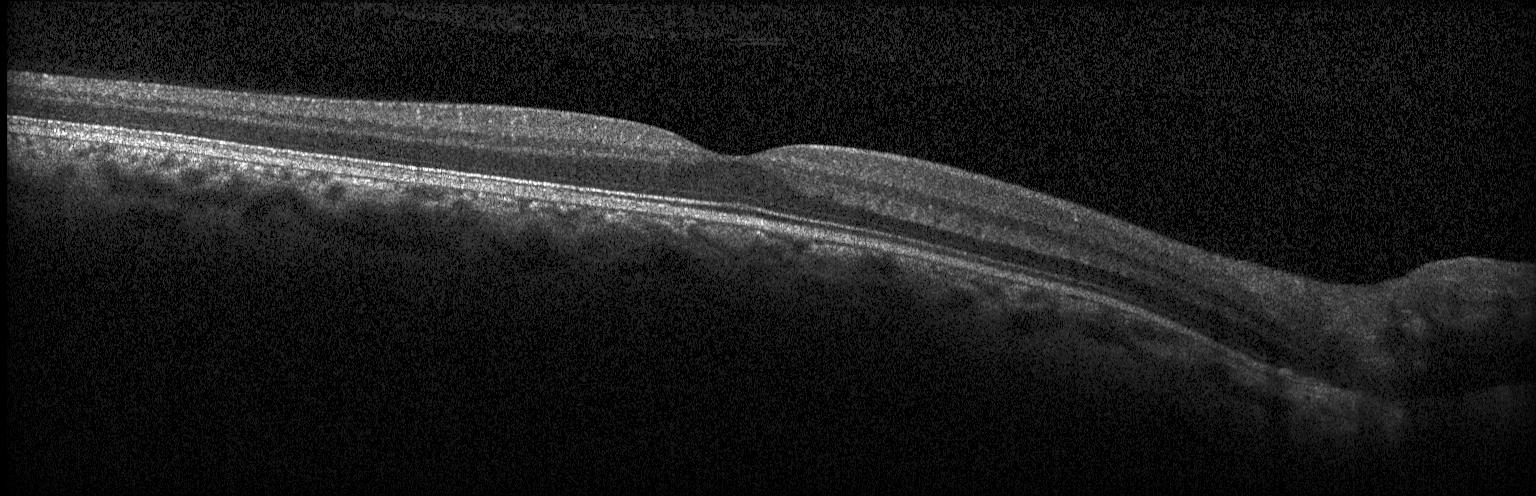
SD-OCT · instrument: Heidelberg Spectralis · optical coherence tomography scan.
No CNV, DME, or drusen.